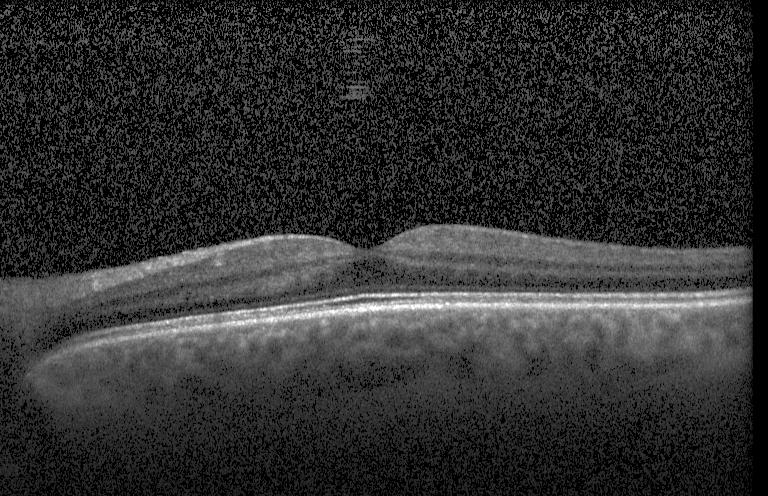 OCT B-scan; instrument: Heidelberg Spectralis; spectral-domain optical coherence tomography. OCT finding: no evidence of choroidal neovascularization, diabetic macular edema, or drusen.